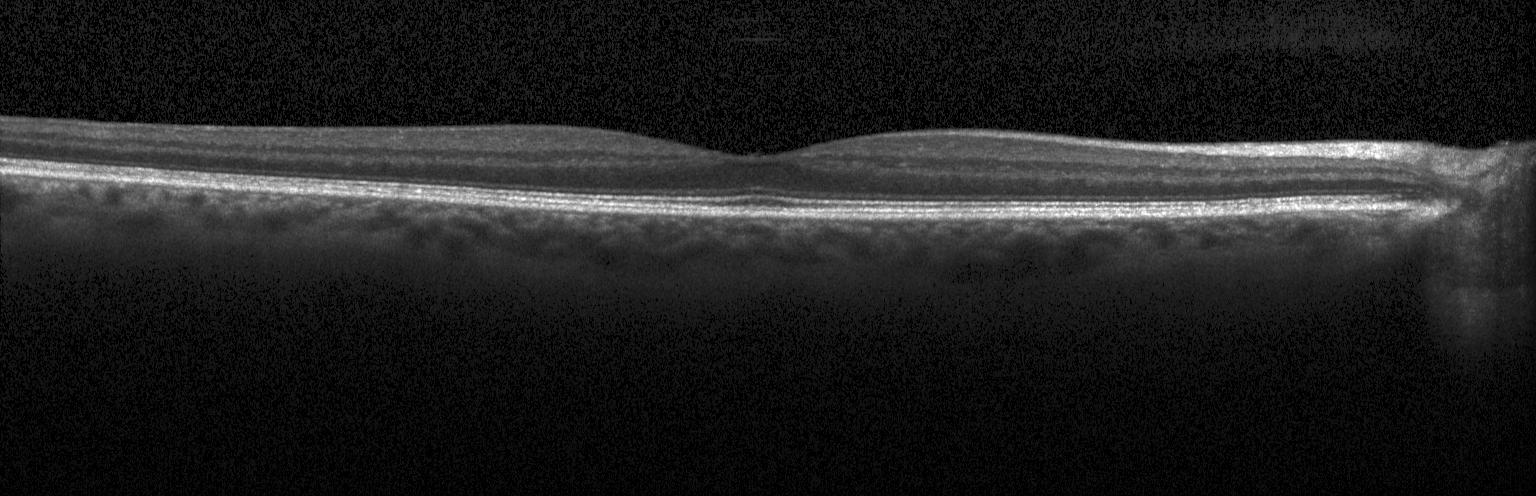 OCT line scan; spectral-domain optical coherence tomography; through the macula; acquired on a Heidelberg Spectralis.
Finding: no choroidal neovascularization, diabetic macular edema, or drusen.